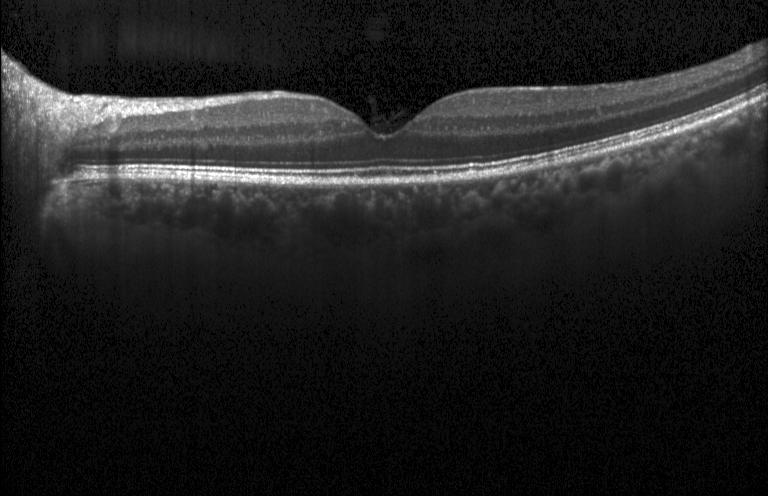
OCT B-scan showing no choroidal neovascularization, diabetic macular edema, or drusen.